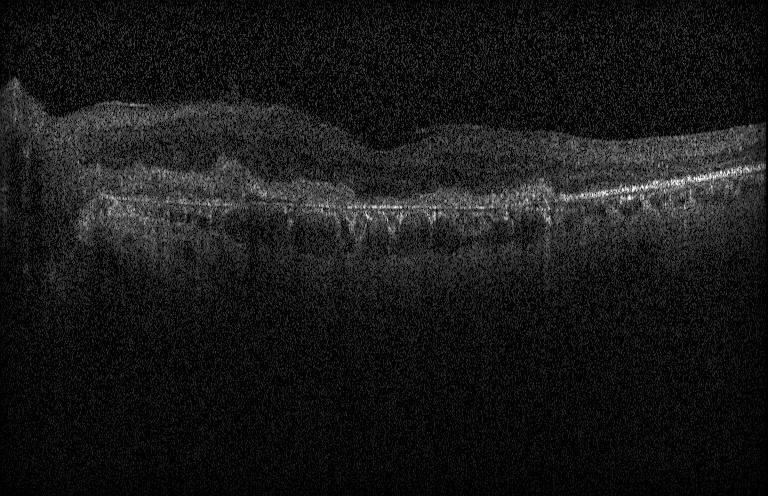
Through the macula · SD-OCT · retinal OCT cross-section · acquired on a Heidelberg Spectralis.
This B-scan demonstrates a choroidal neovascular membrane.